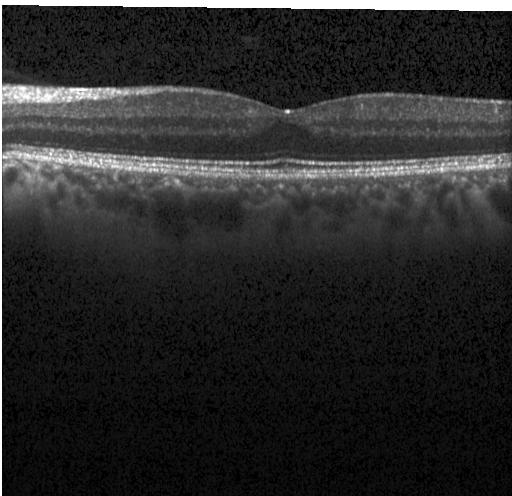
Retinal OCT cross-section. SD-OCT. Finding: no choroidal neovascularization, no diabetic macular edema, and no drusen.